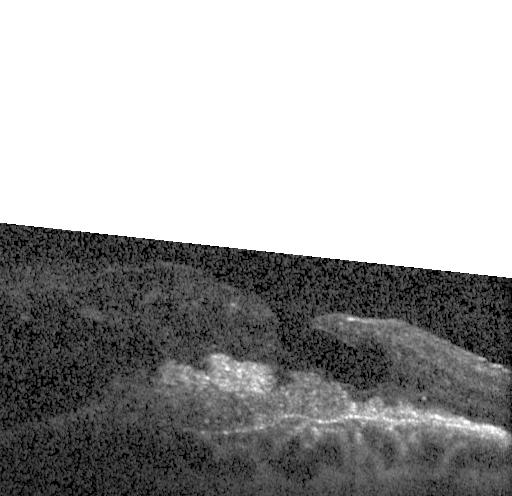
Instrument: Heidelberg Spectralis, OCT B-scan
Impression: choroidal neovascularization.